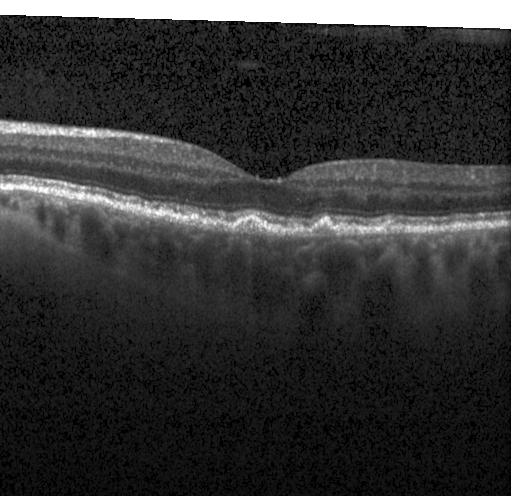

Assessment: multiple drusen.